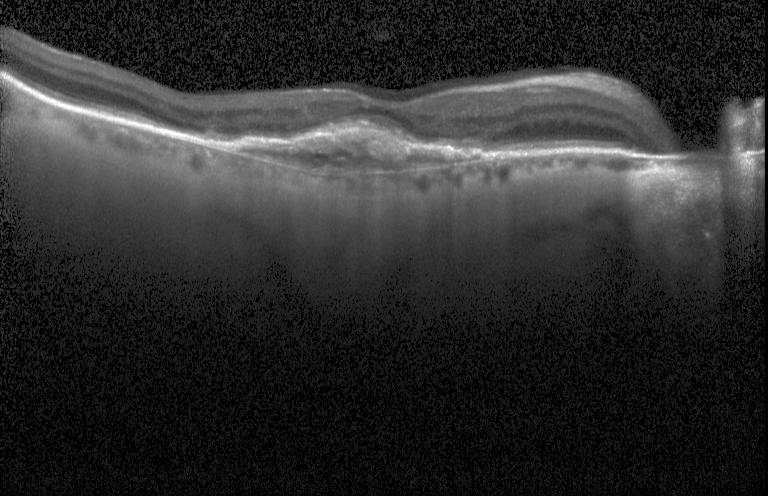
Centered on the fovea · optical coherence tomography scan · spectral-domain OCT
Macular OCT: choroidal neovascularization.